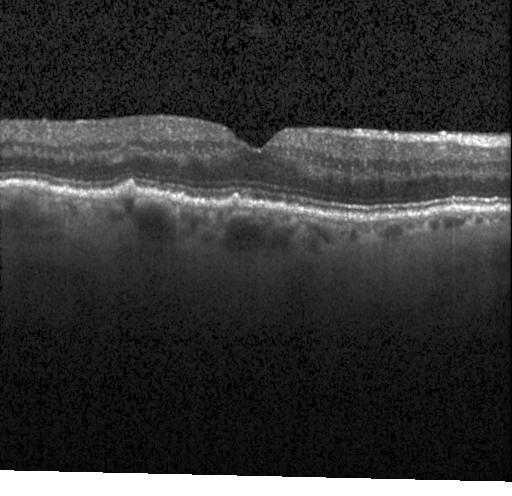 Macular OCT: multiple drusen.